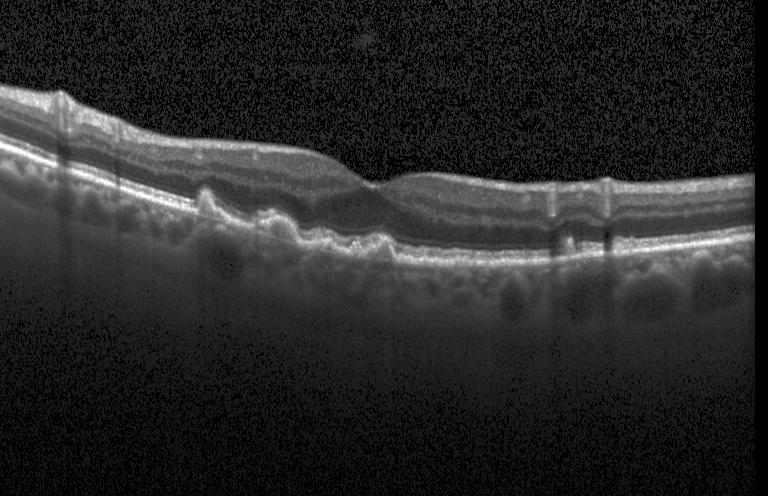

Through the macula, optical coherence tomography B-scan, Heidelberg Spectralis OCT system — Diagnosis: drusen.